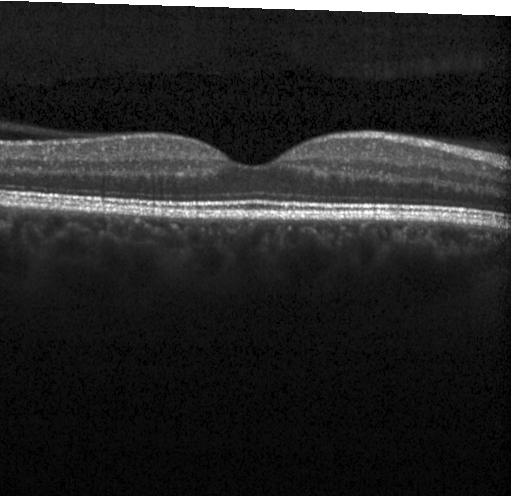
Macular OCT demonstrating no CNV, no DME, and no drusen.